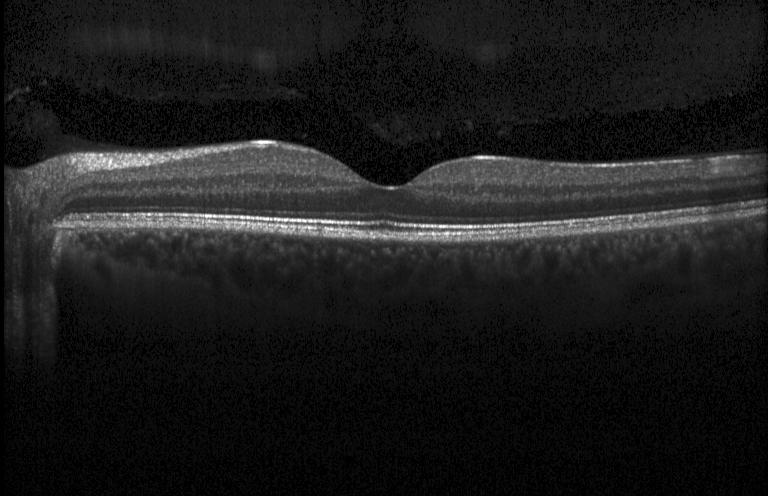 OCT B-scan. The scan shows no choroidal neovascularization, diabetic macular edema, or drusen.